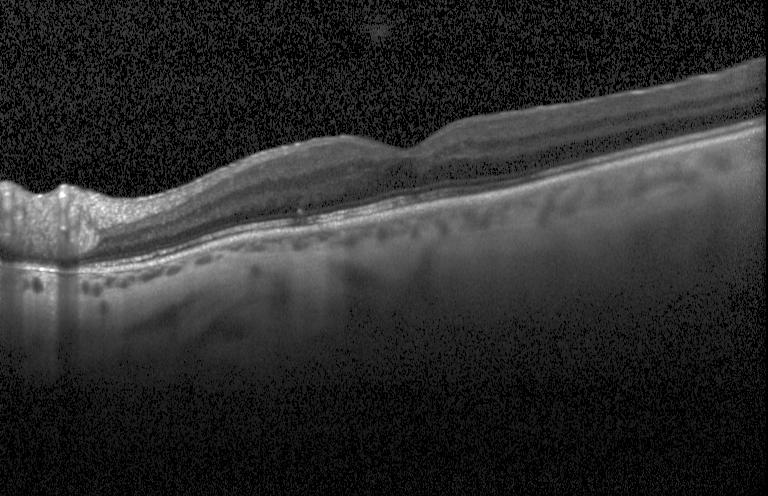
Heidelberg Spectralis · optical coherence tomography scan.
The scan shows no evidence of choroidal neovascularization, diabetic macular edema, or drusen.